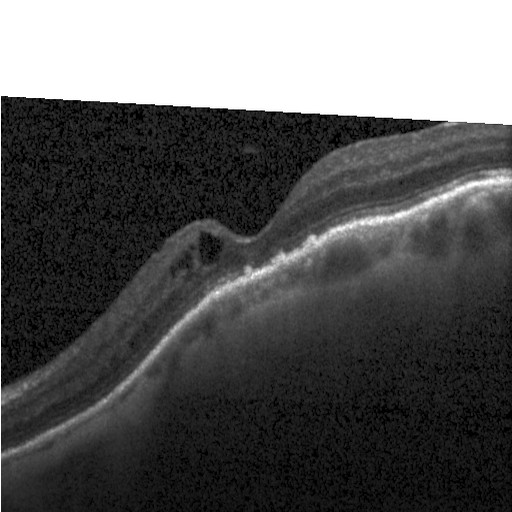
Impression: DME.